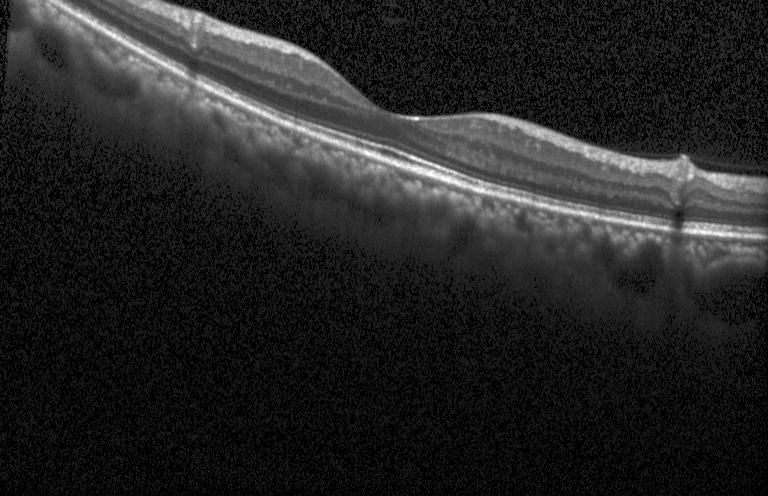
OCT B-scan — Diagnosis: no CNV, no DME, and no drusen.